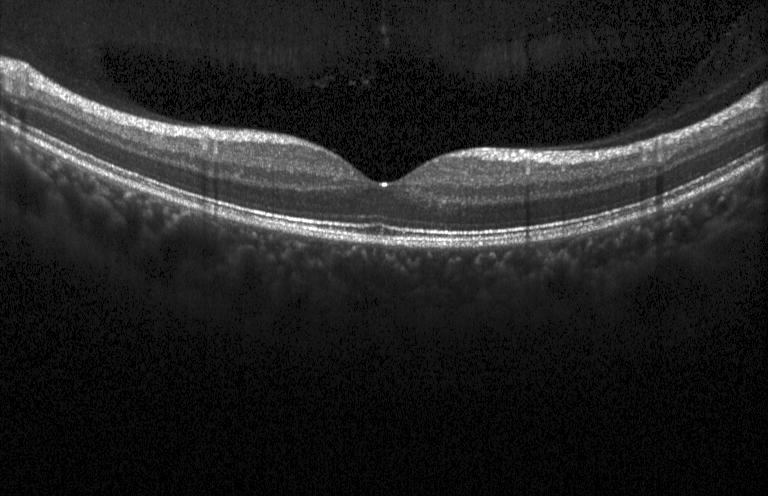 Optical coherence tomography B-scan · Heidelberg Spectralis
Diagnosis: no choroidal neovascularization, diabetic macular edema, or drusen.